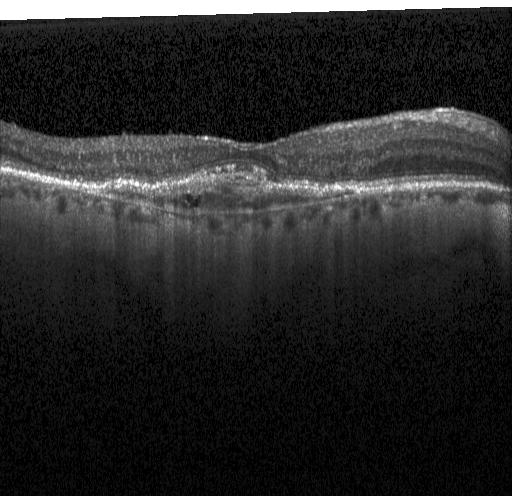

Retinal OCT cross-section showing a choroidal neovascular membrane.